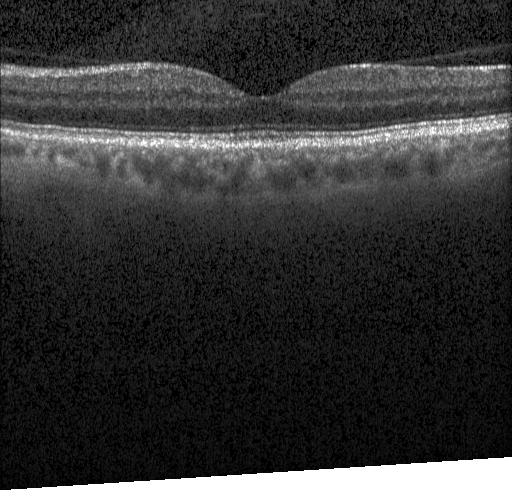
Diagnosis: no choroidal neovascularization, diabetic macular edema, or drusen.